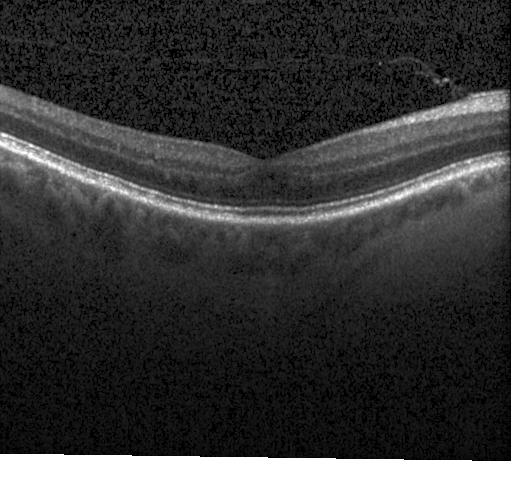

Fovea-centered · retinal OCT B-scan
This B-scan demonstrates neither choroidal neovascularization, diabetic macular edema, nor drusen.